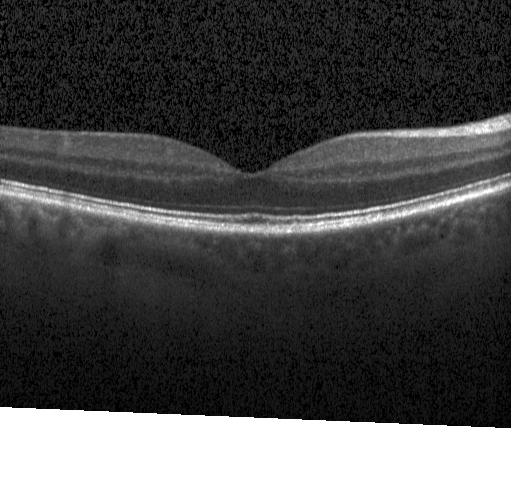

No evidence of choroidal neovascularization, diabetic macular edema, or drusen.